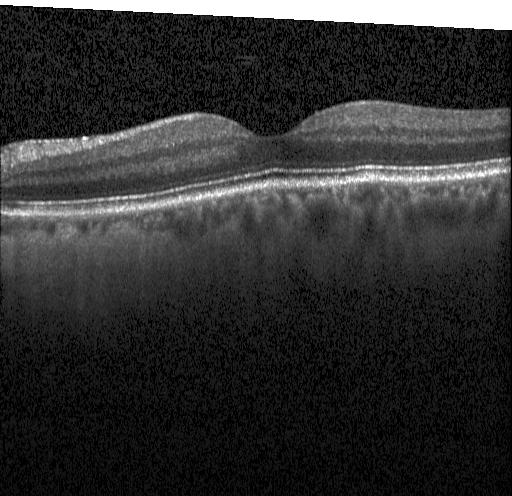

OCT scan showing neither choroidal neovascularization, diabetic macular edema, nor drusen.